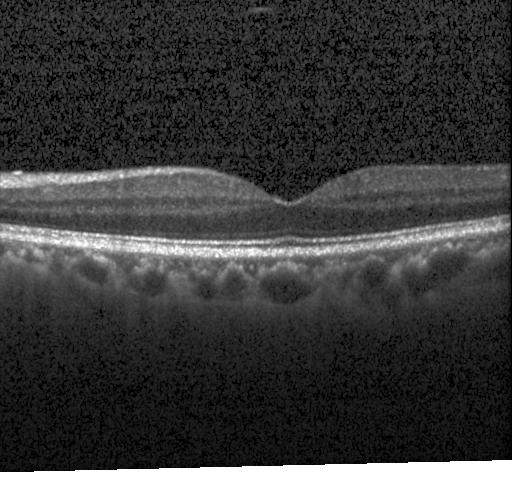
Impression: neither CNV, DME, nor drusen.